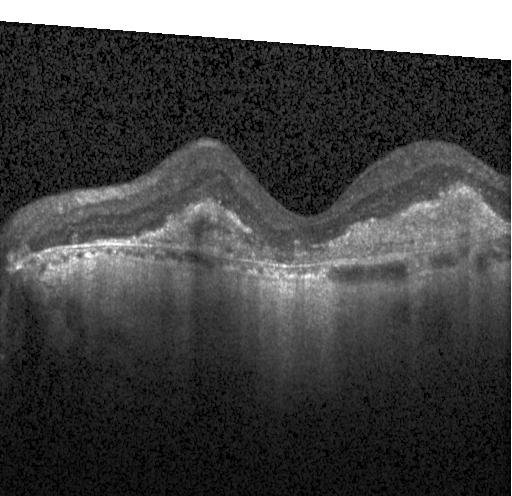

Centered on the fovea; spectral-domain optical coherence tomography; instrument: Heidelberg Spectralis; OCT B-scan. Finding: CNV.